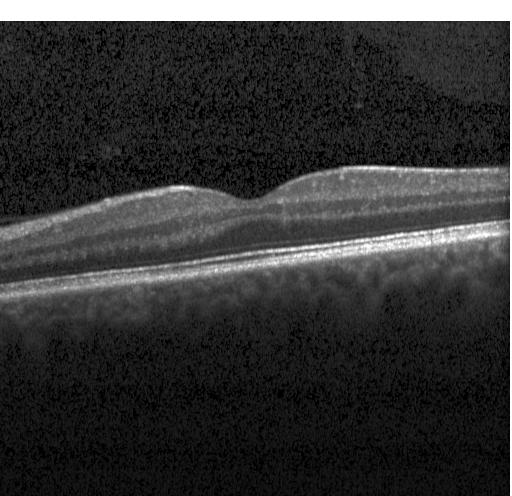 Through the macula; retinal OCT cross-section. Finding: no choroidal neovascularization, diabetic macular edema, or drusen.